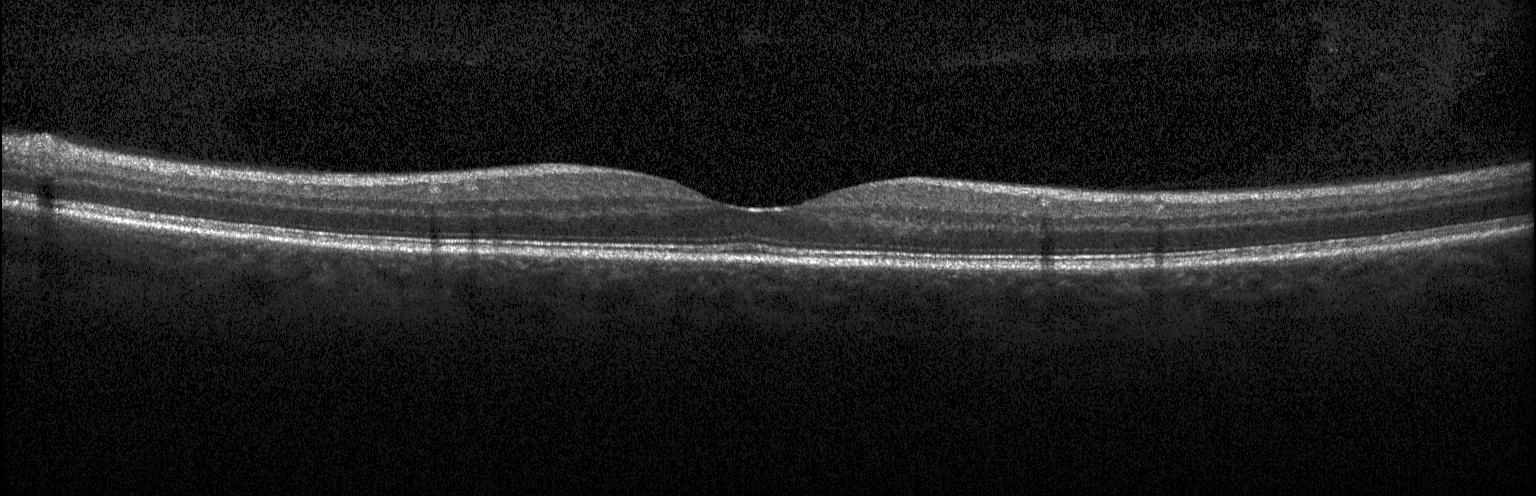

Diagnosis: neither CNV, DME, nor drusen.